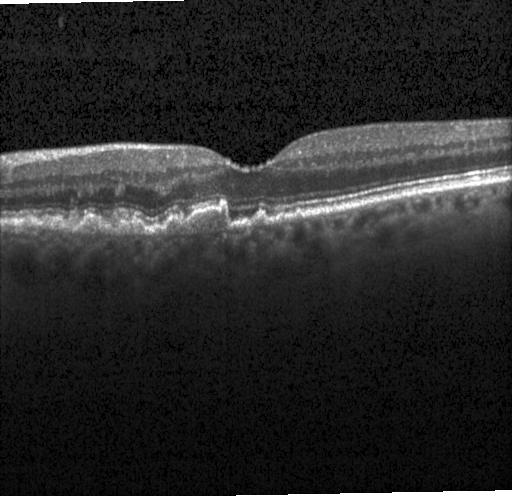

The scan shows drusen.